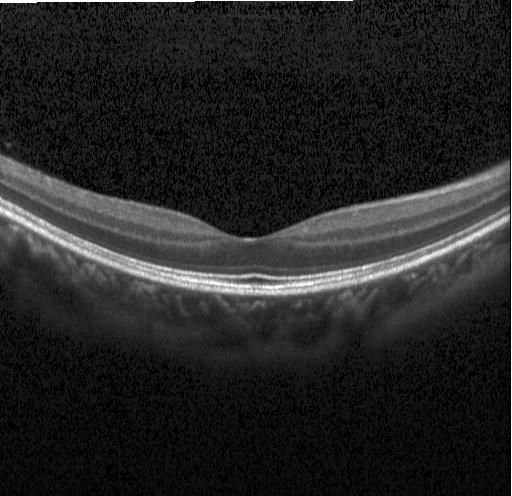 Optical coherence tomography B-scan. Heidelberg Spectralis OCT system — This B-scan demonstrates no CNV, DME, or drusen.